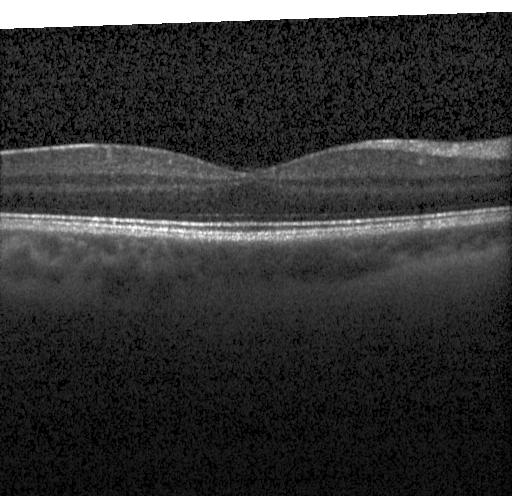
Spectral-domain OCT, OCT line scan, horizontal scan through the fovea
Diagnosis: neither CNV, DME, nor drusen.